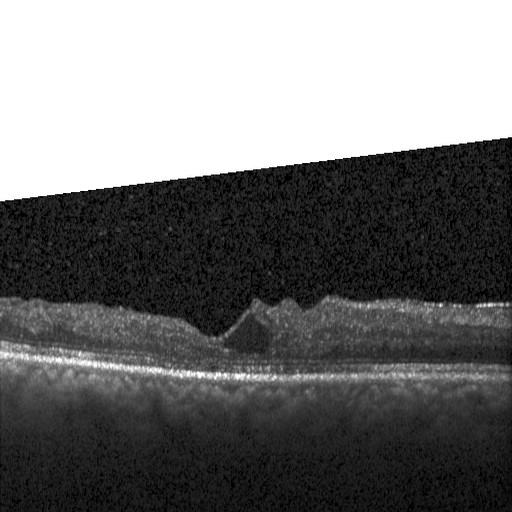
Spectral-domain OCT B-scan: diabetic macular edema.